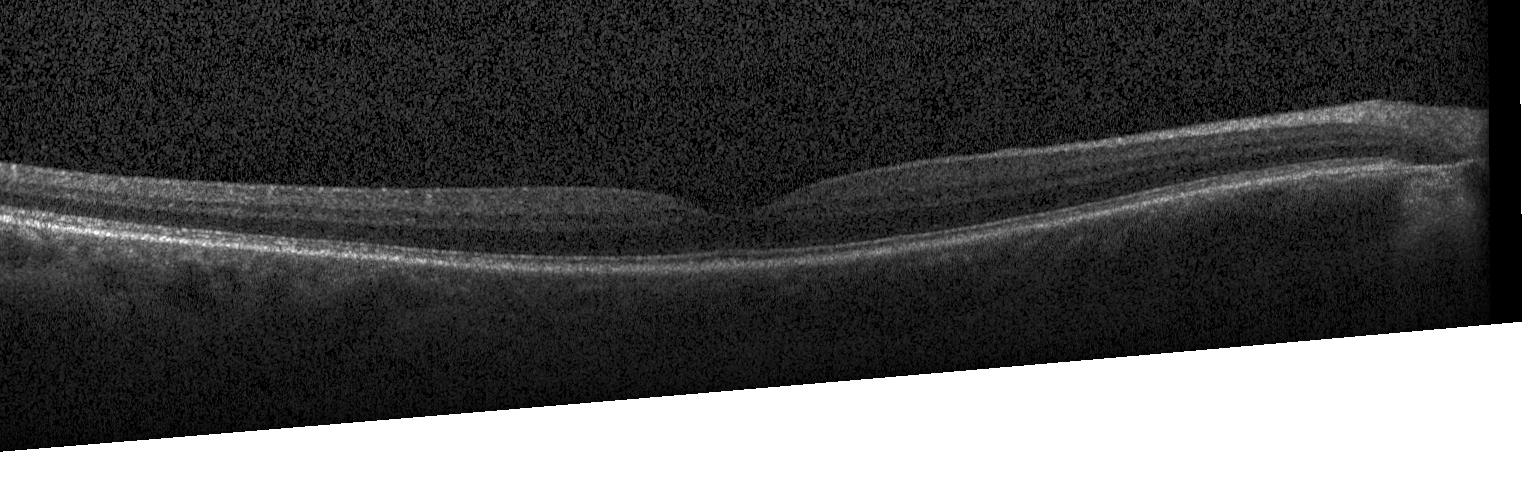

Diagnosis: no choroidal neovascularization, no diabetic macular edema, and no drusen.